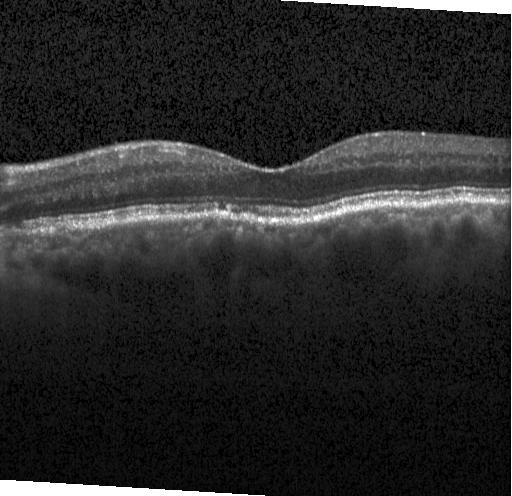 Spectral-domain OCT B-scan: neither choroidal neovascularization, diabetic macular edema, nor drusen.